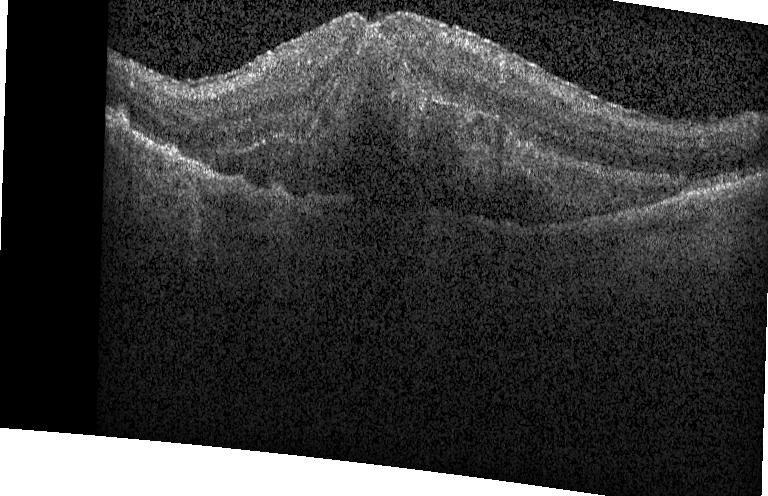

Diagnosis: choroidal neovascularization (CNV).